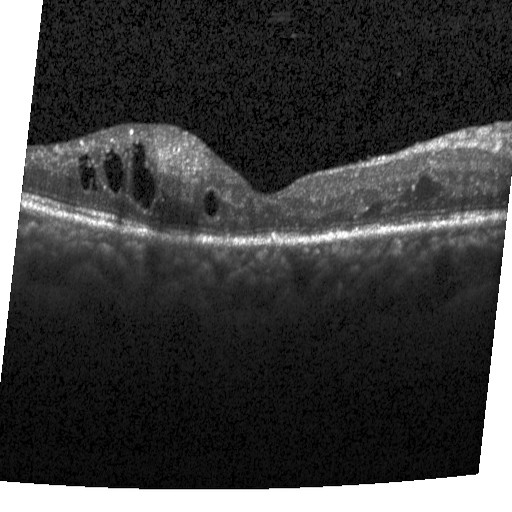 Spectral-domain optical coherence tomography, through the macula, acquired on a Heidelberg Spectralis, optical coherence tomography B-scan
Impression: diabetic macular edema (DME).